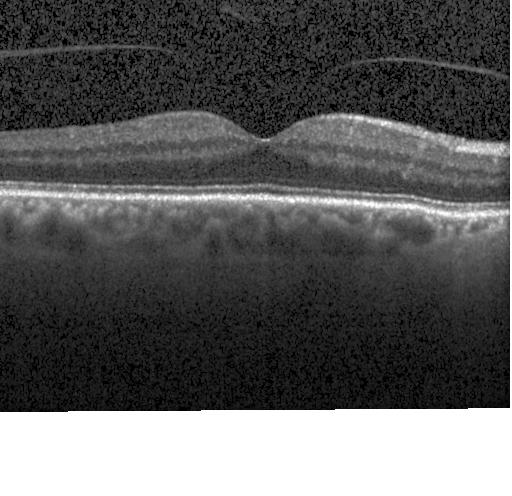 Impression: no choroidal neovascularization, diabetic macular edema, or drusen.